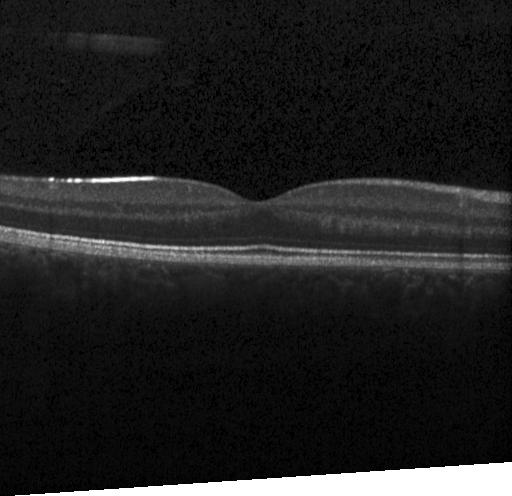
Horizontal scan through the fovea, SD-OCT, OCT line scan, Heidelberg Spectralis
Dx: no evidence of choroidal neovascularization, diabetic macular edema, or drusen.